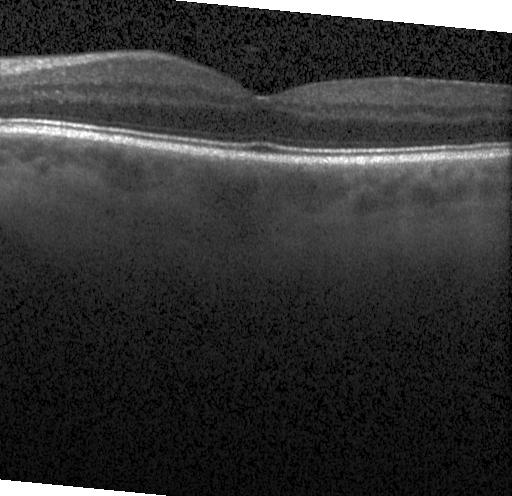

Retinal OCT B-scan, macular scan. Macular OCT: no choroidal neovascularization, no diabetic macular edema, and no drusen.